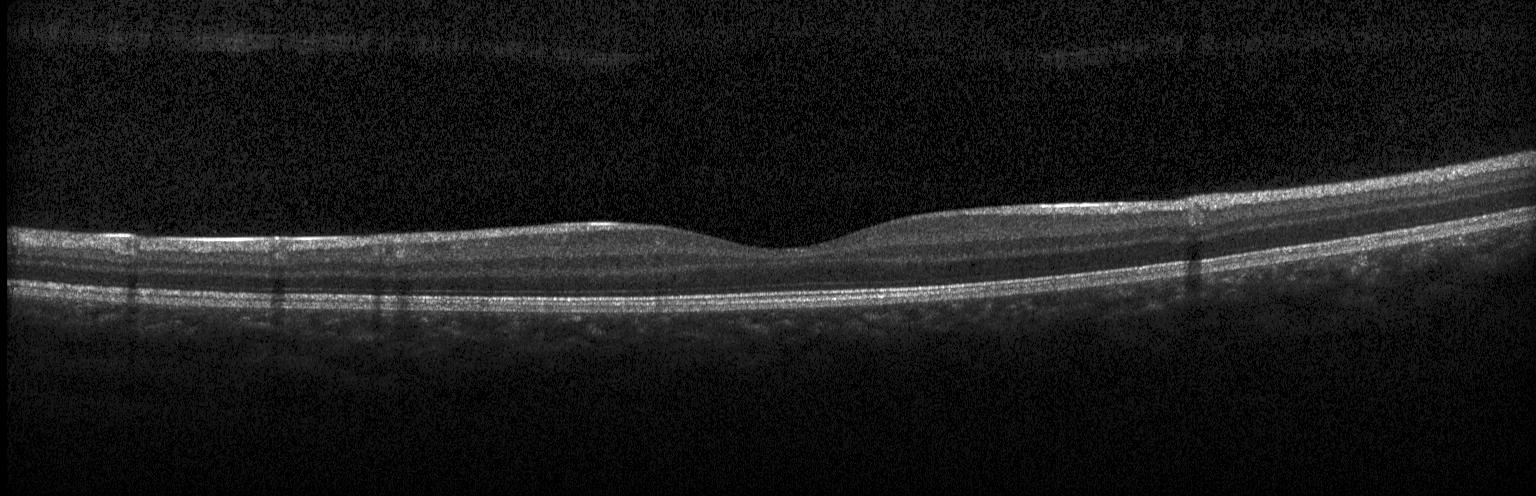 Spectral-domain OCT, retinal OCT cross-section, centered on the fovea, acquired on a Heidelberg Spectralis
Macular OCT: no CNV, no DME, and no drusen.